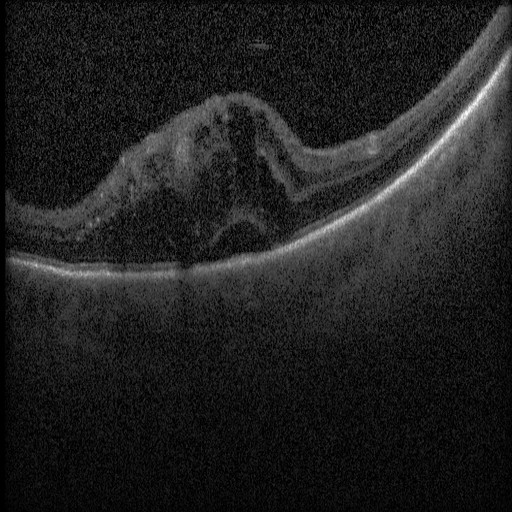 Optical coherence tomography B-scan. Spectral-domain OCT. Fovea-centered. DME.